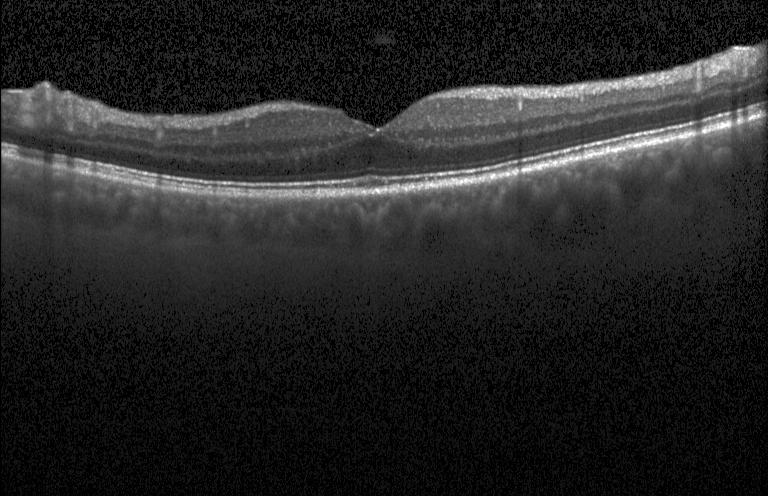
Diagnosis: no CNV, no DME, and no drusen.